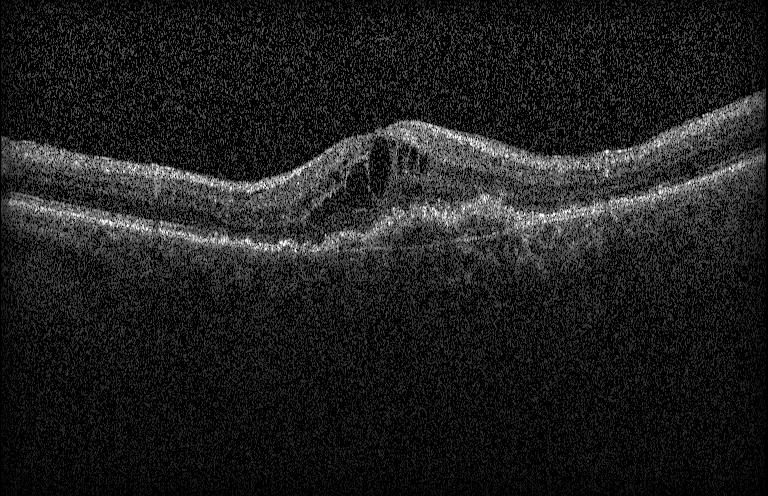
Retinal OCT cross-section. Instrument: Heidelberg Spectralis. CNV.